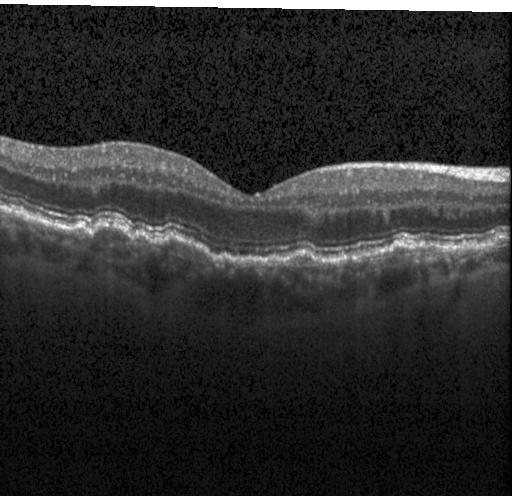 Impression: drusen.